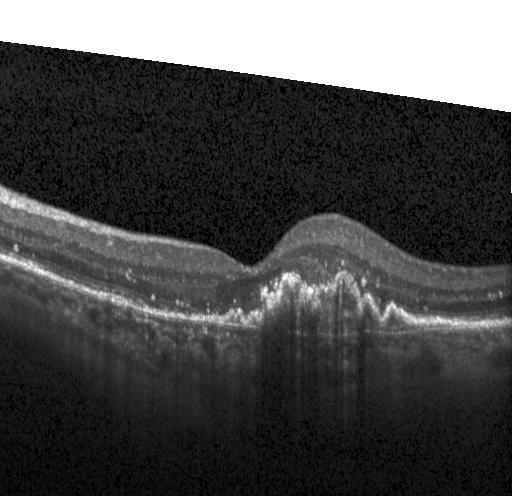

Retinal OCT cross-section · macular scan · Heidelberg Spectralis OCT system
The scan shows a choroidal neovascular membrane.